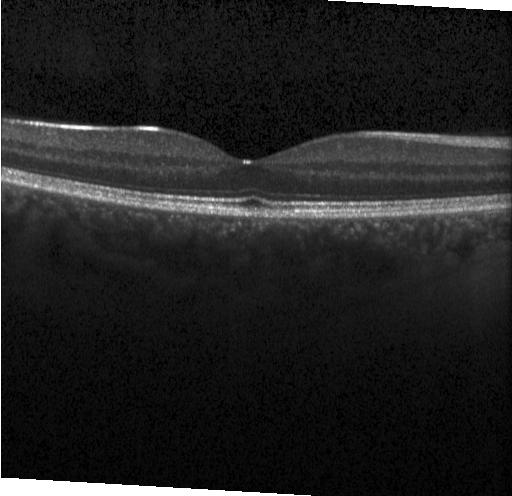 Retinal OCT B-scan
OCT finding: no CNV, no DME, and no drusen.